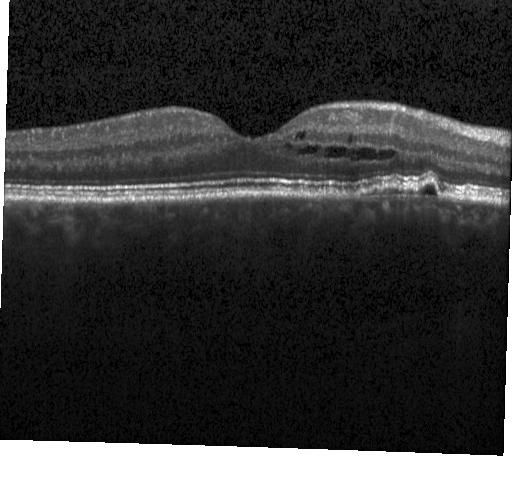
OCT B-scan, Heidelberg Spectralis OCT system, spectral-domain OCT, centered on the fovea
Diagnosis: a choroidal neovascular membrane.